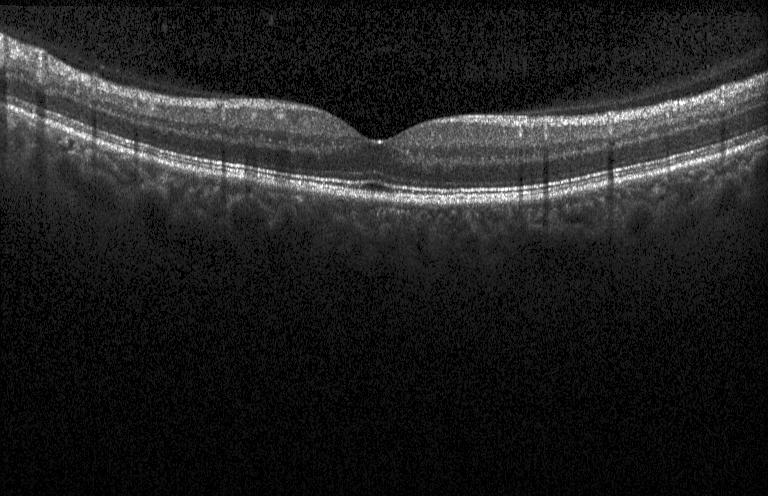

The scan shows no choroidal neovascularization, diabetic macular edema, or drusen.